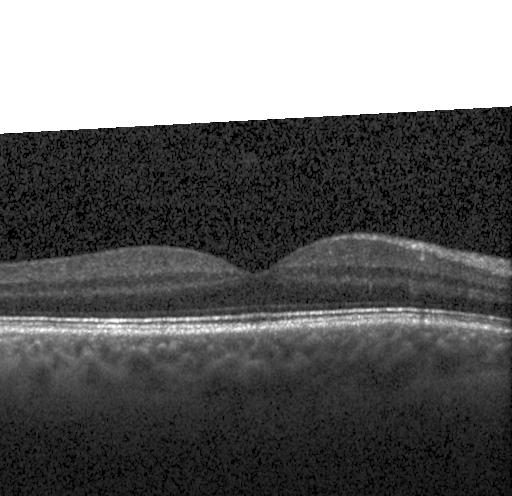

Finding: no evidence of choroidal neovascularization, diabetic macular edema, or drusen.